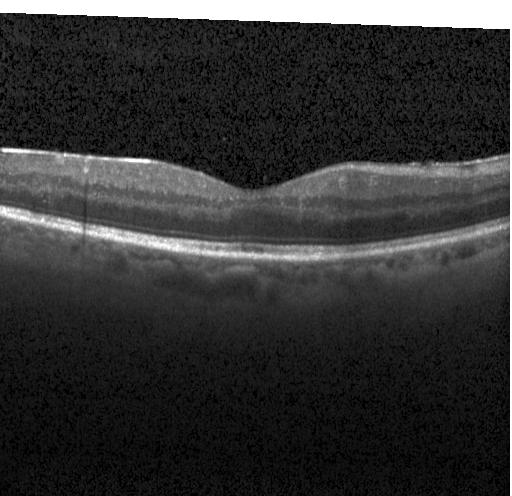 Neither CNV, DME, nor drusen.